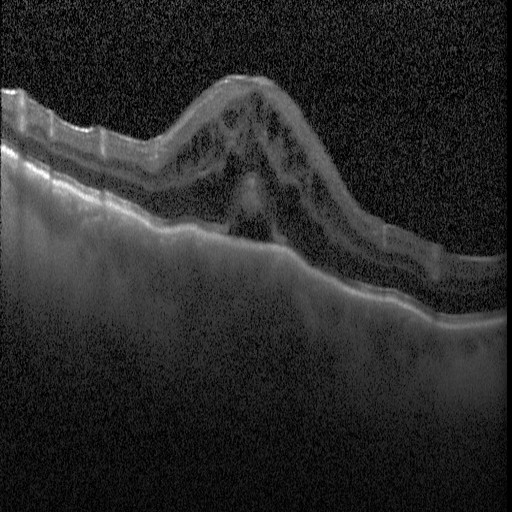

Optical coherence tomography scan; SD-OCT
Diagnosis: diabetic macular edema.